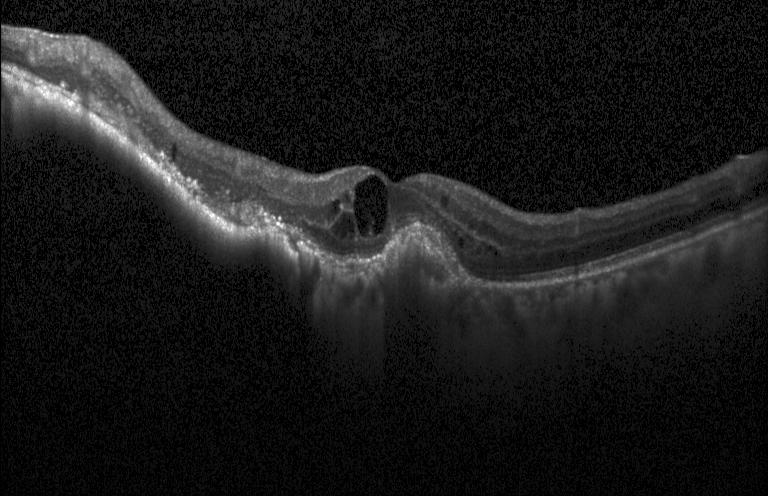 This B-scan demonstrates a choroidal neovascular membrane.